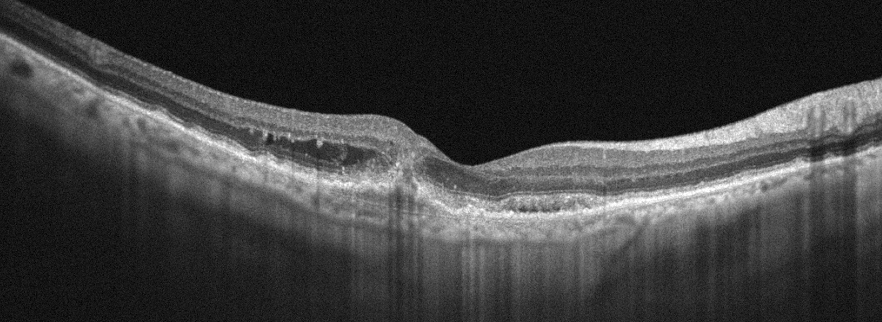
This B-scan demonstrates age-related macular degeneration (AMD).